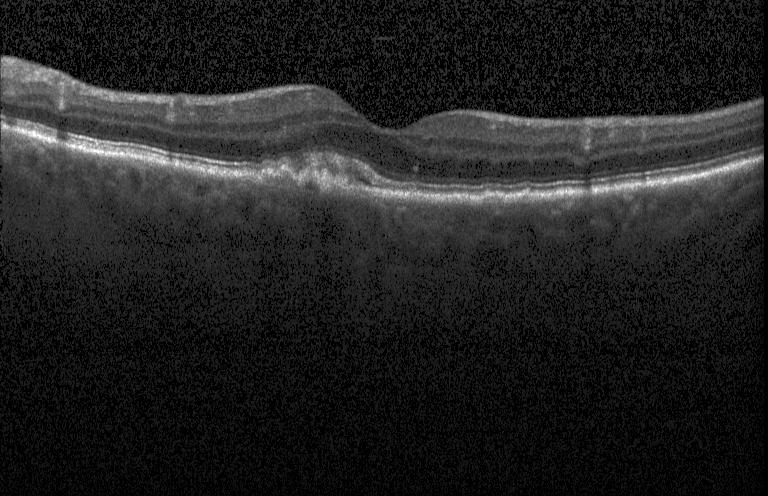

Heidelberg Spectralis, retinal OCT cross-section, centered on the fovea
Dx: a choroidal neovascular membrane.